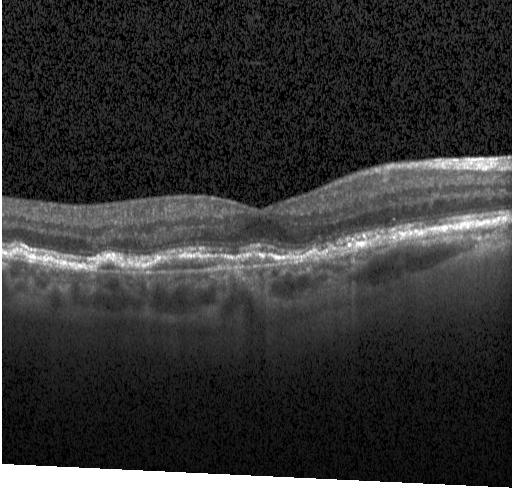
Diagnosis: choroidal neovascularization (CNV).